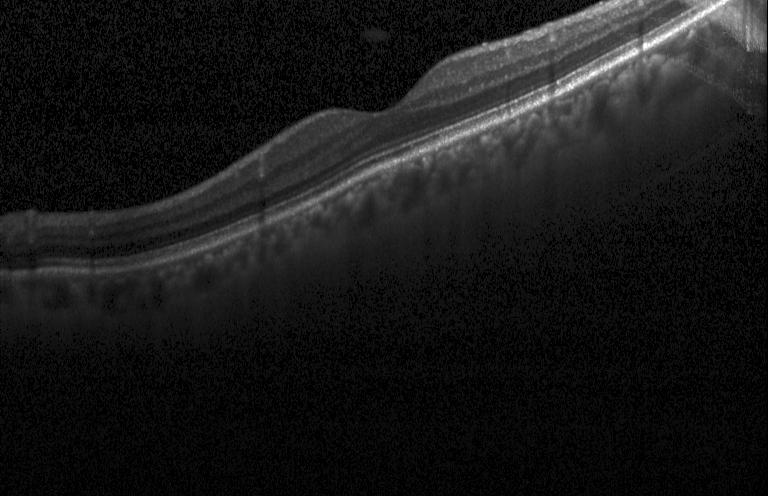 OCT finding: no CNV, DME, or drusen.